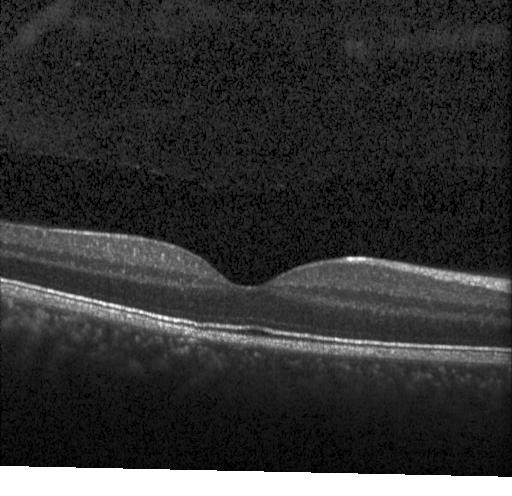 Instrument: Heidelberg Spectralis · SD-OCT · OCT line scan. Diagnosis: no evidence of choroidal neovascularization, diabetic macular edema, or drusen.